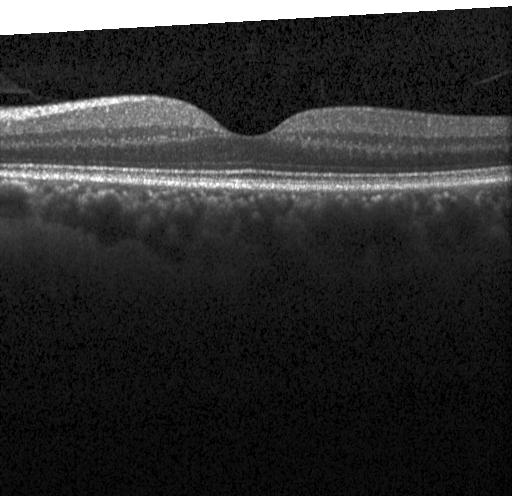

Retinal OCT cross-section — Macular OCT: neither CNV, DME, nor drusen.